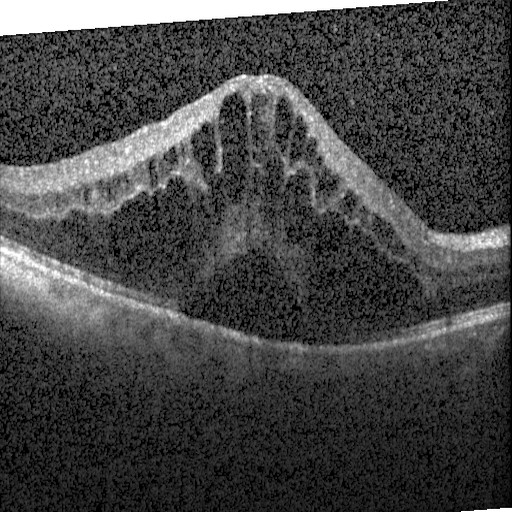

Finding: diabetic macular edema (DME).